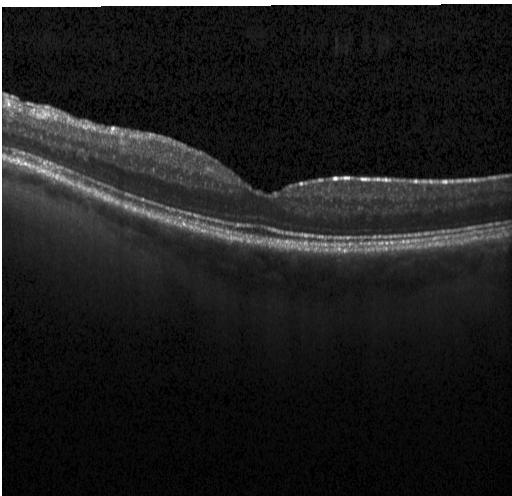
Through the macula. Spectral-domain OCT. Retinal OCT cross-section
Assessment: no CNV, DME, or drusen.